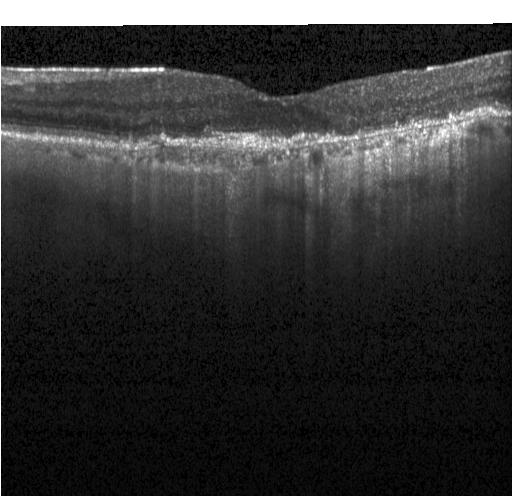

Retinal OCT cross-section showing CNV.